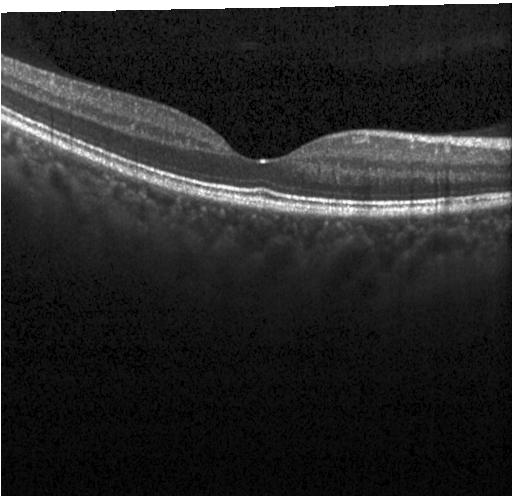 Macular scan. OCT B-scan. Heidelberg Spectralis OCT system — Diagnosis: no CNV, DME, or drusen.